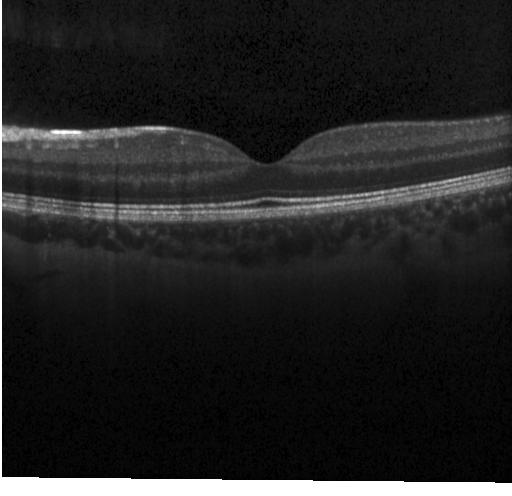
OCT scan showing no evidence of CNV, DME, or drusen.